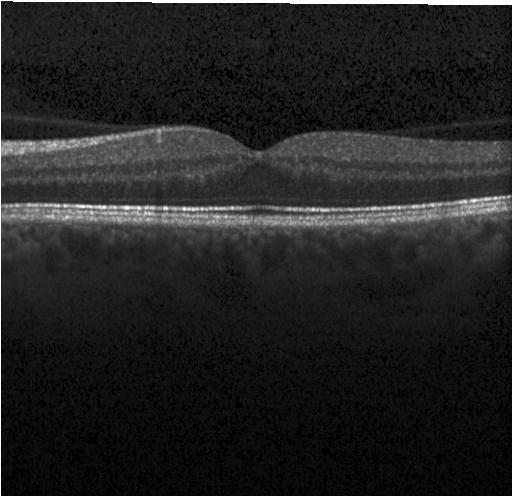
Retinal OCT cross-section.
The scan shows no CNV, DME, or drusen.